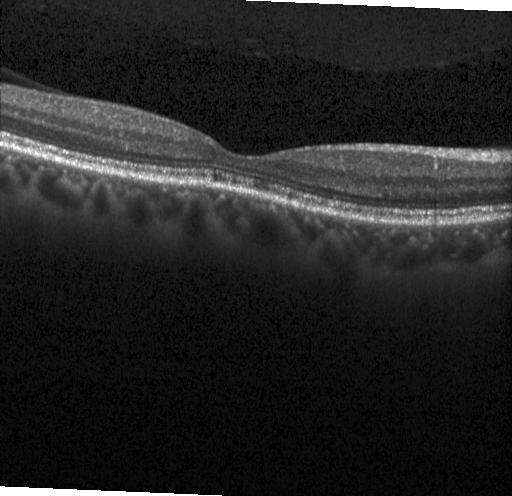 OCT finding: neither choroidal neovascularization, diabetic macular edema, nor drusen.